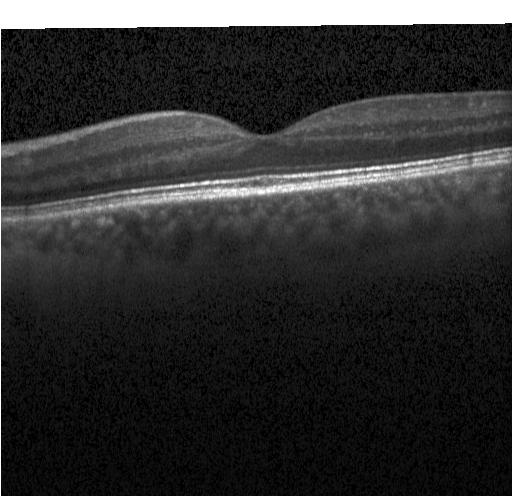

The scan shows no evidence of choroidal neovascularization, diabetic macular edema, or drusen.